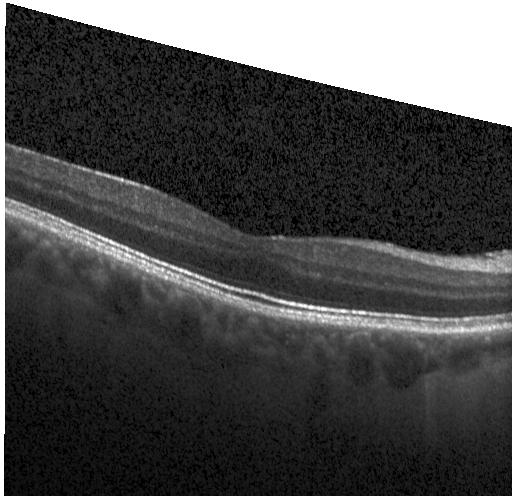
Spectral-domain OCT; retinal OCT cross-section.
Assessment: no CNV, DME, or drusen.